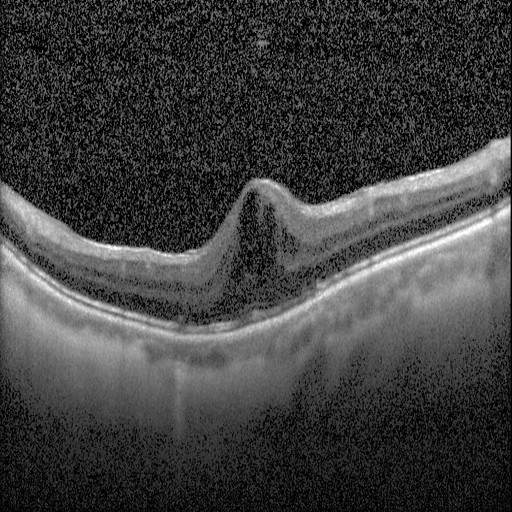 Retinal OCT cross-section. SD-OCT. Horizontal scan through the fovea. Heidelberg Spectralis OCT system — This B-scan demonstrates diabetic macular edema.